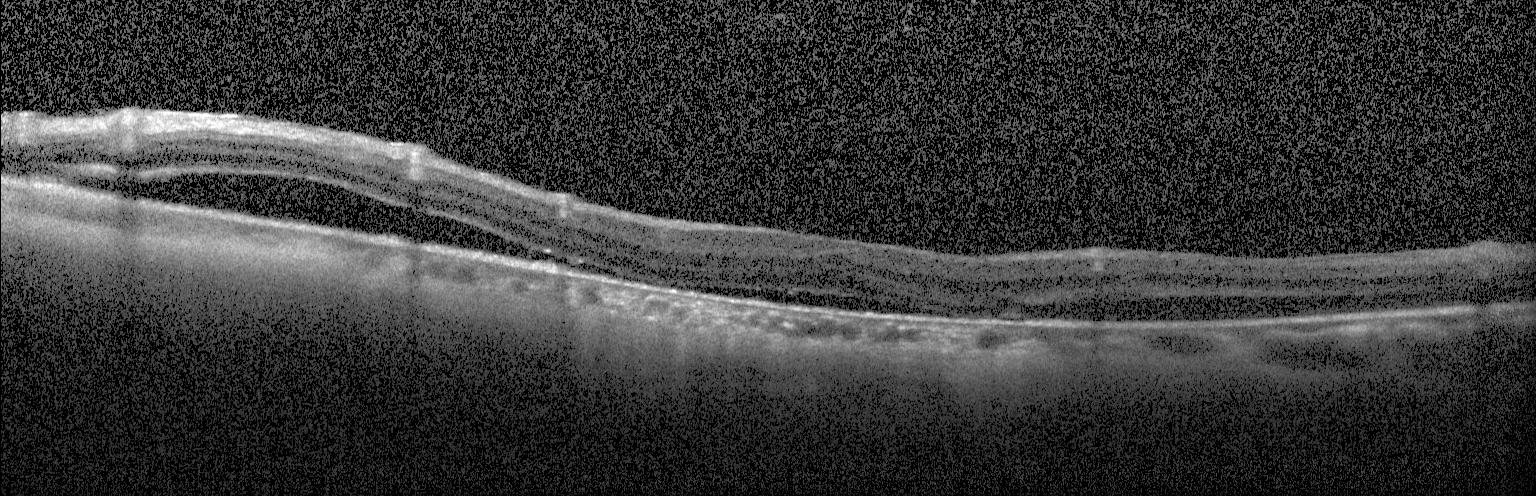
Acquired on a Heidelberg Spectralis. OCT B-scan. Centered on the fovea. Impression: CNV.